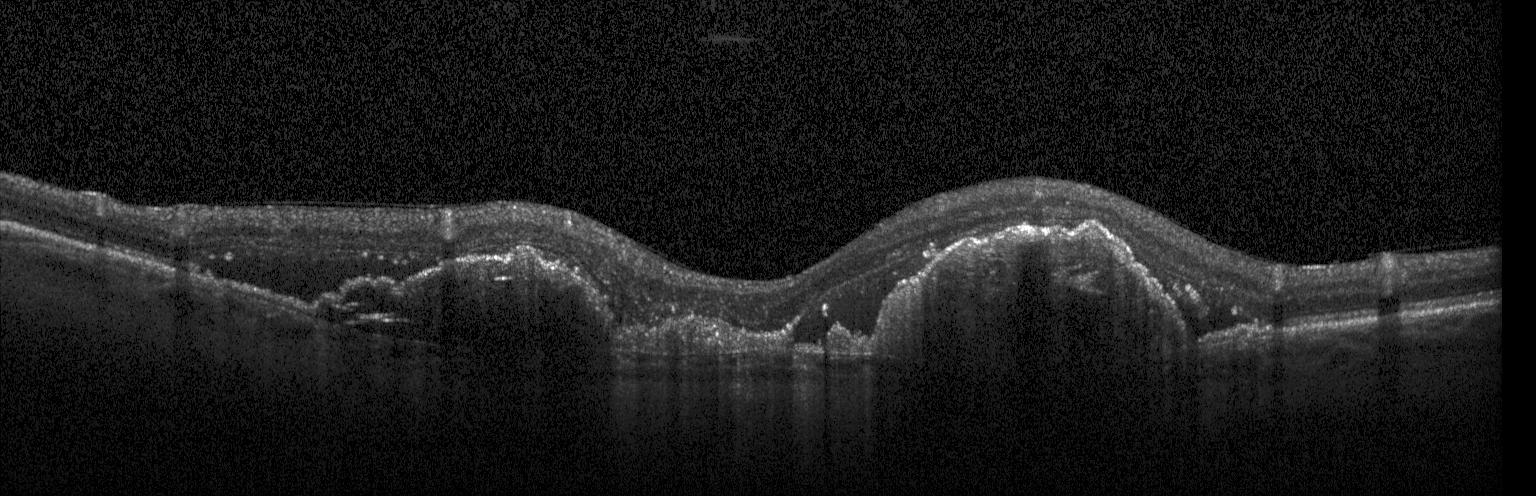 Diagnosis: CNV.